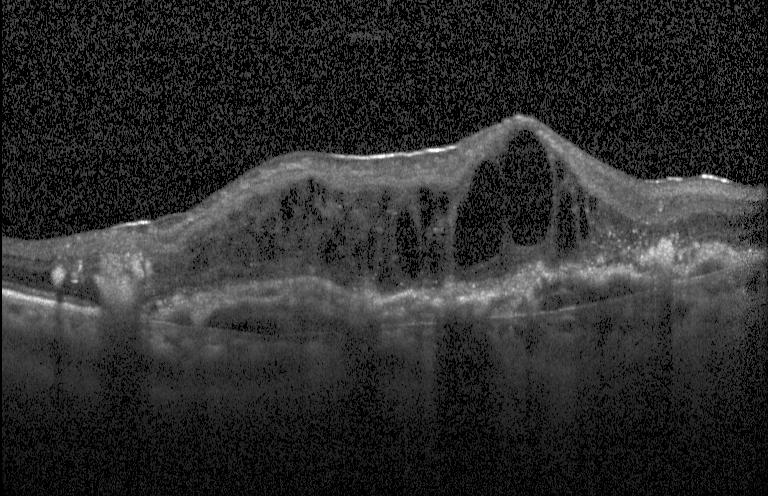 Horizontal scan through the fovea; OCT B-scan. Assessment: a choroidal neovascular membrane.